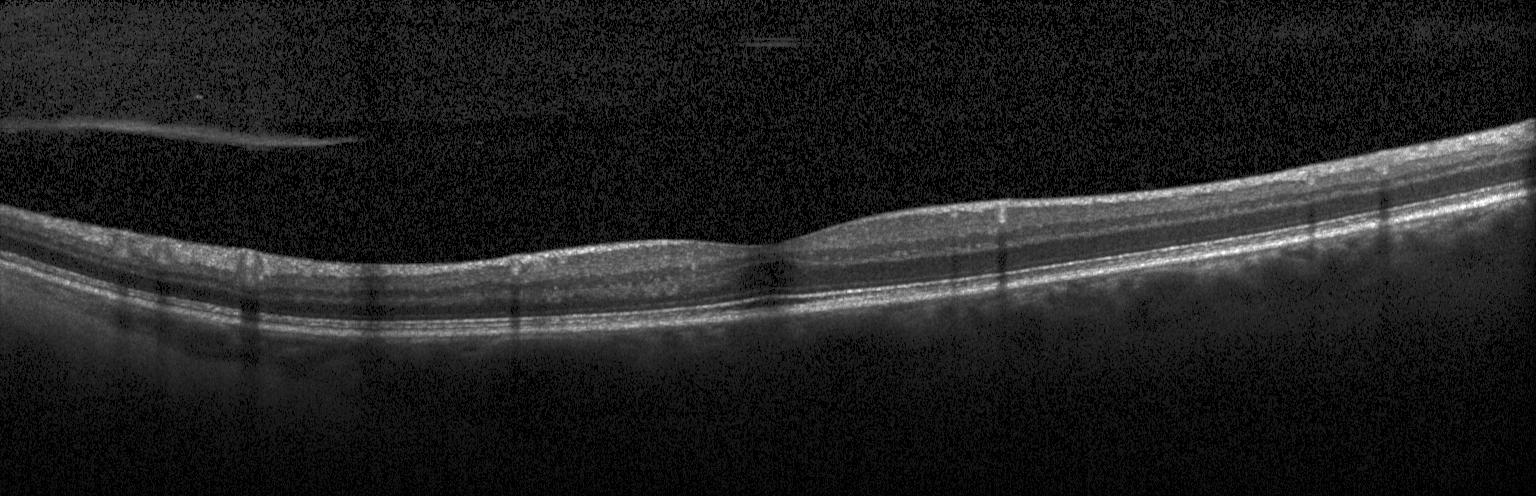

Macular OCT demonstrating neither CNV, DME, nor drusen.